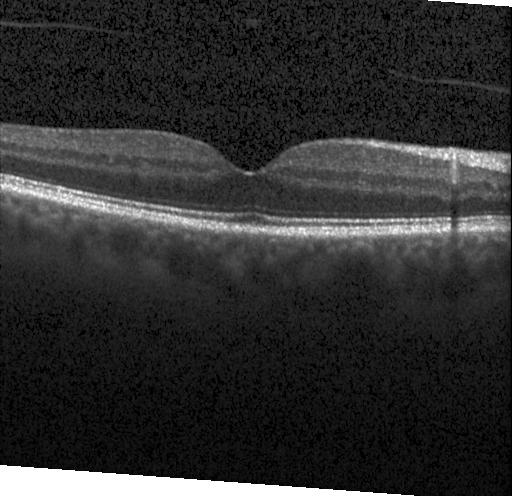 Macular OCT demonstrating no CNV, no DME, and no drusen.